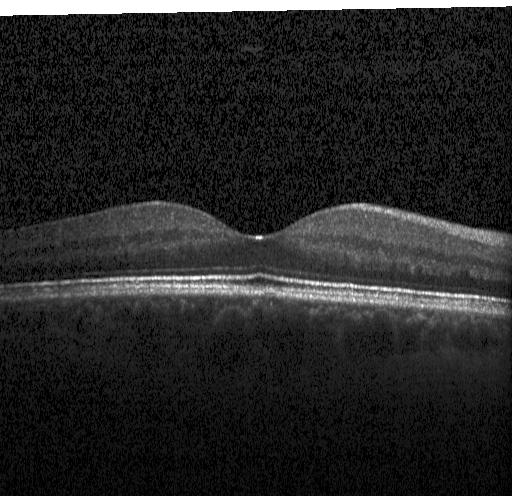

Horizontal scan through the fovea · spectral-domain OCT · Heidelberg Spectralis OCT system · optical coherence tomography B-scan.
Dx: no choroidal neovascularization, no diabetic macular edema, and no drusen.